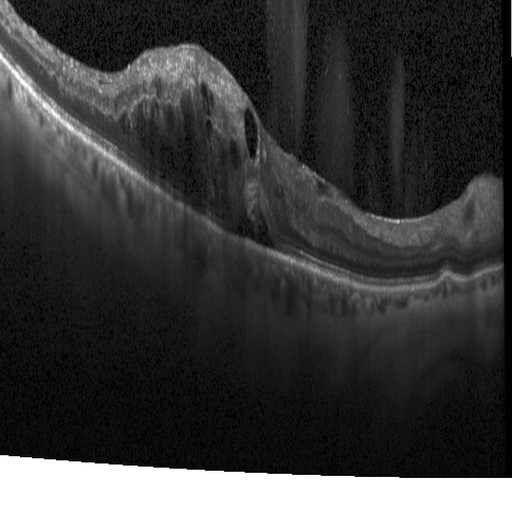

Diagnosis: DME.